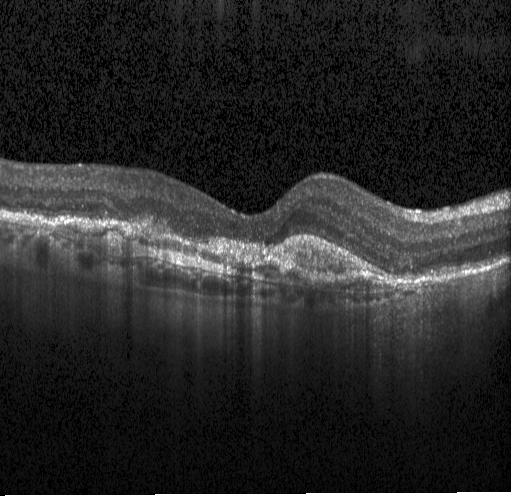 Macular scan, spectral-domain OCT, Heidelberg Spectralis, OCT line scan.
Finding: choroidal neovascularization (CNV).